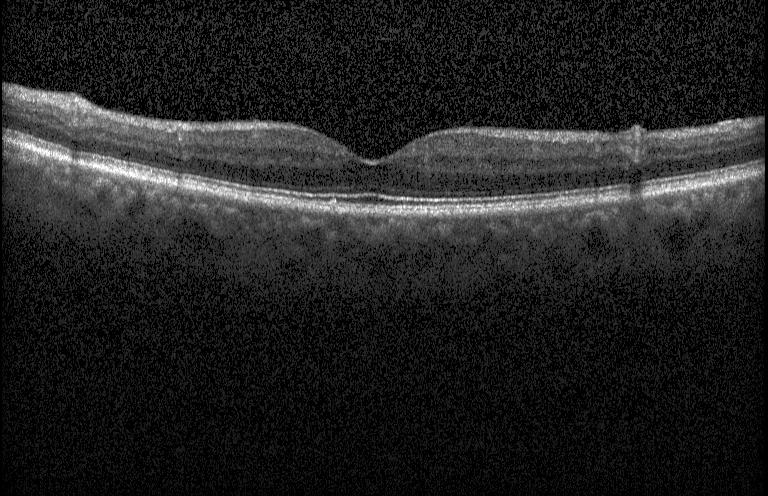 OCT line scan, SD-OCT, macular scan, instrument: Heidelberg Spectralis — Diagnosis: no CNV, DME, or drusen.